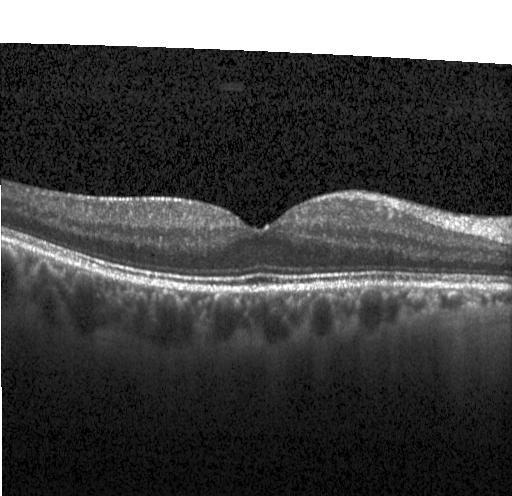 Dx: no evidence of CNV, DME, or drusen.